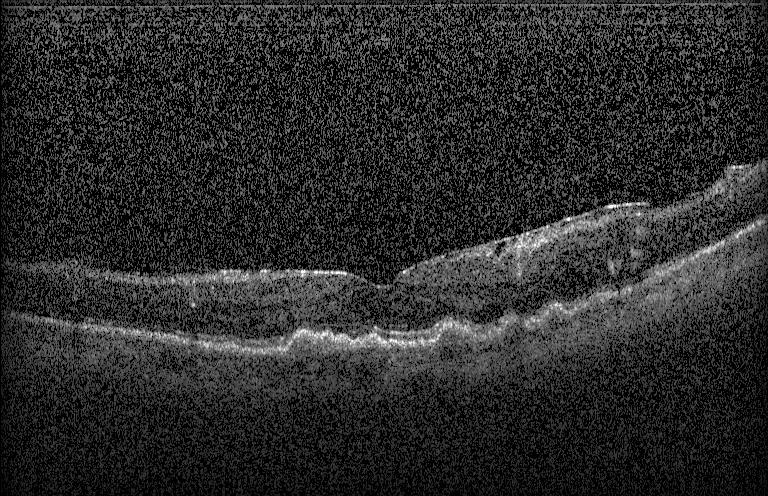
Diagnosis: drusen.